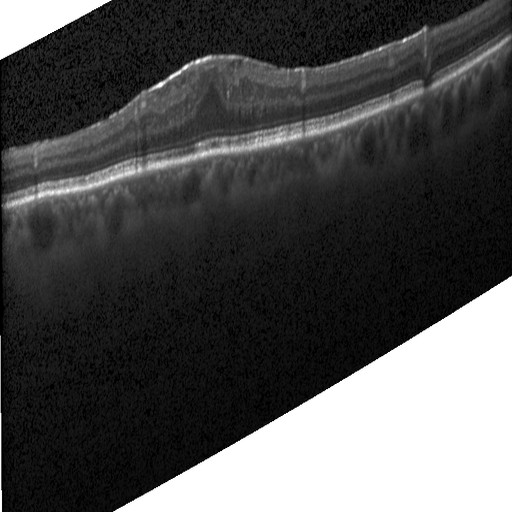 DME.